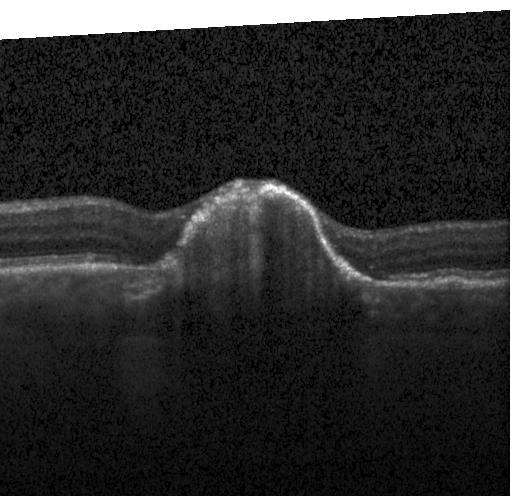

OCT B-scan. Impression: a choroidal neovascular membrane.